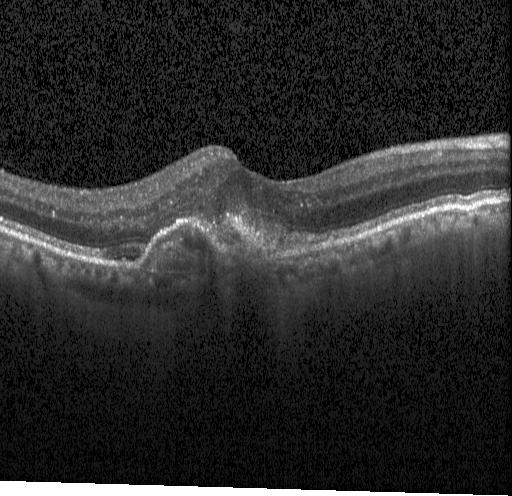
Diagnosis: a choroidal neovascular membrane.